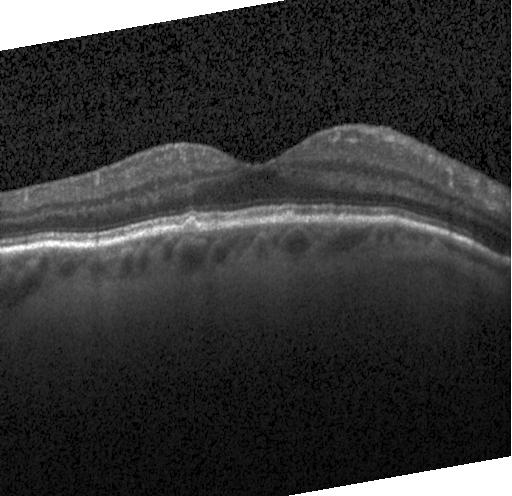

Centered on the fovea. Retinal OCT B-scan.
This B-scan demonstrates multiple drusen.